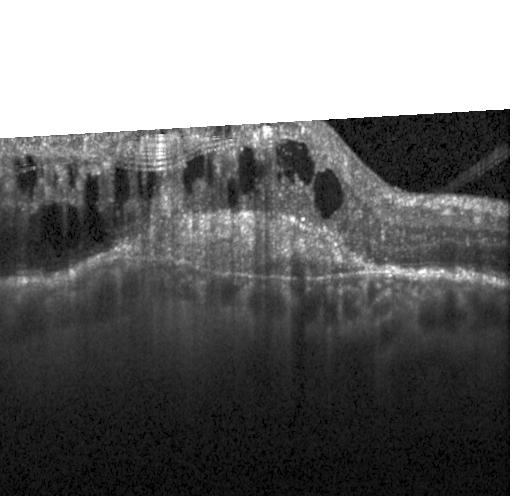

Instrument: Heidelberg Spectralis, spectral-domain optical coherence tomography, OCT line scan — Diagnosis: choroidal neovascularization (CNV).